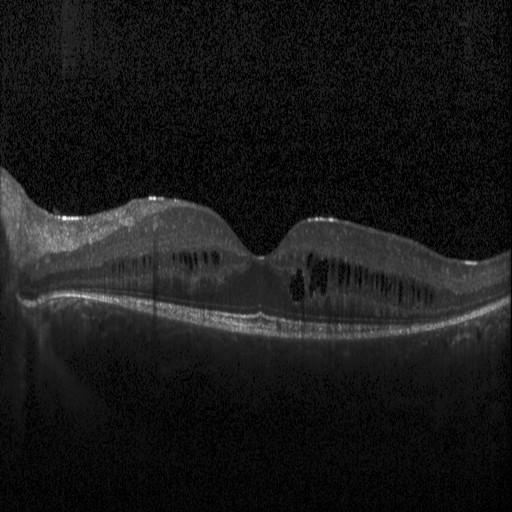 Impression: diabetic macular edema (DME).